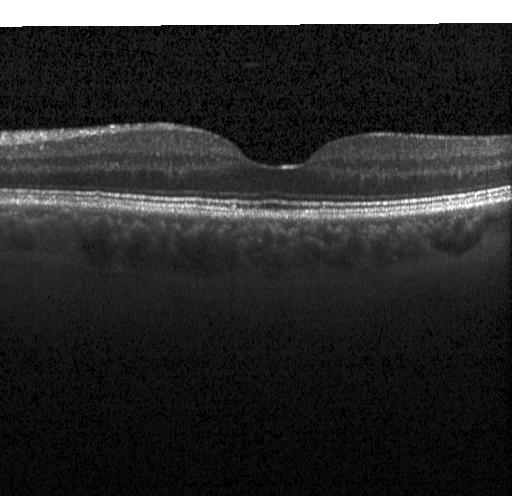 No evidence of choroidal neovascularization, diabetic macular edema, or drusen.